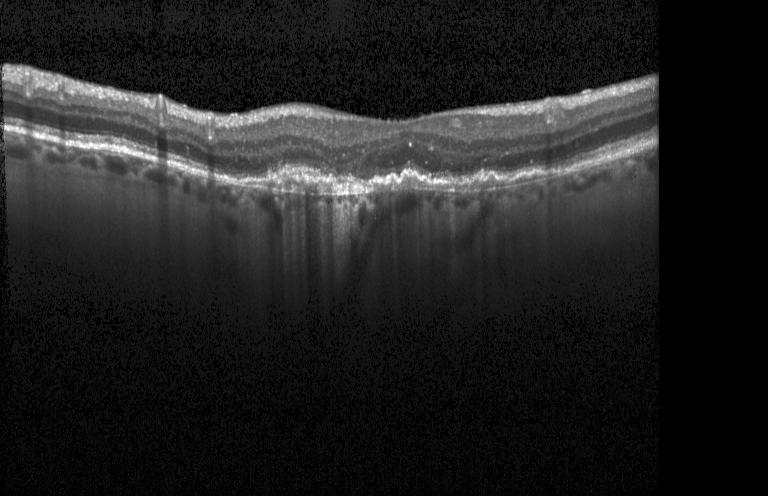

OCT B-scan — Assessment: a choroidal neovascular membrane.